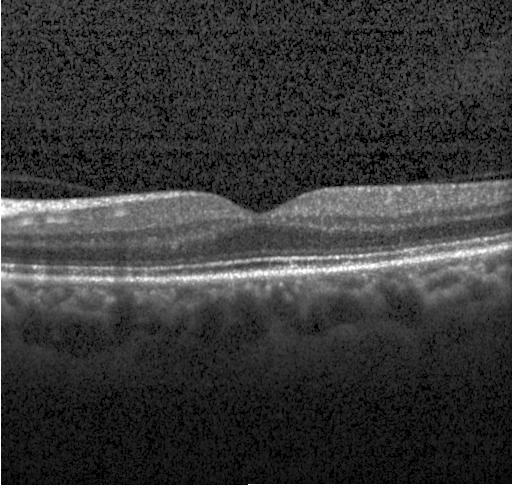

OCT line scan. Through the macula. SD-OCT
The scan shows neither choroidal neovascularization, diabetic macular edema, nor drusen.